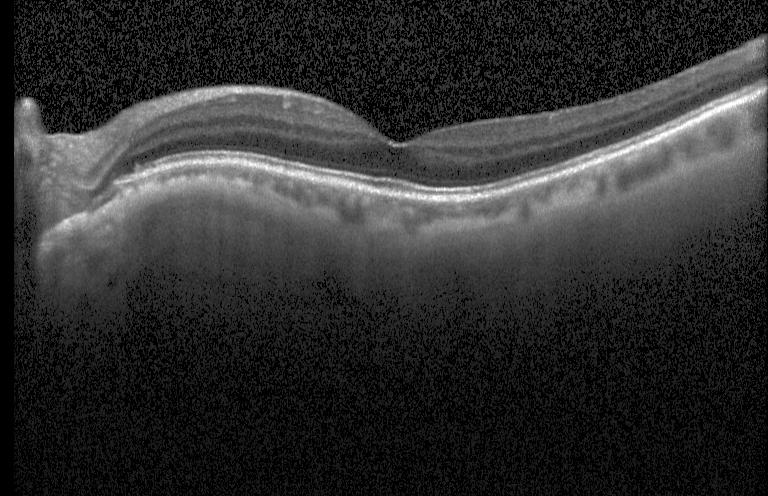

This B-scan demonstrates neither choroidal neovascularization, diabetic macular edema, nor drusen.